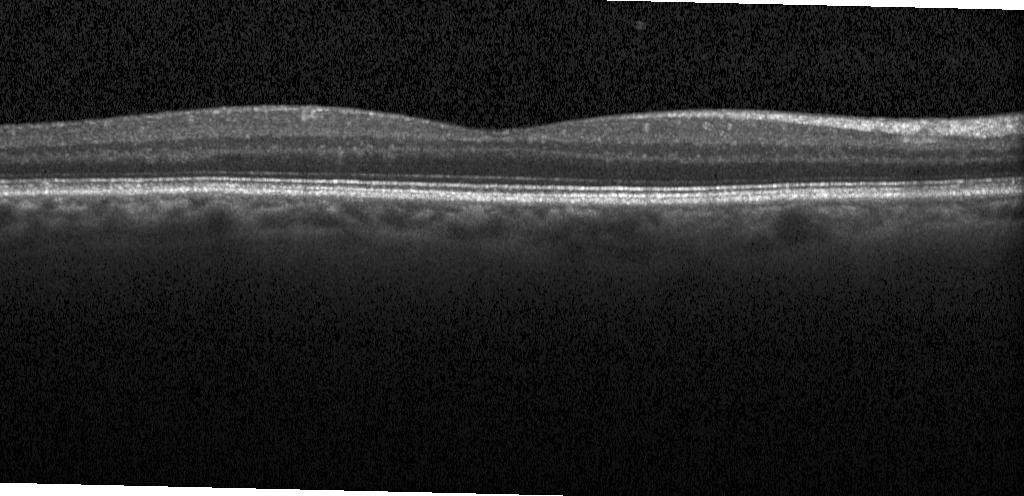

OCT line scan
This B-scan demonstrates neither choroidal neovascularization, diabetic macular edema, nor drusen.